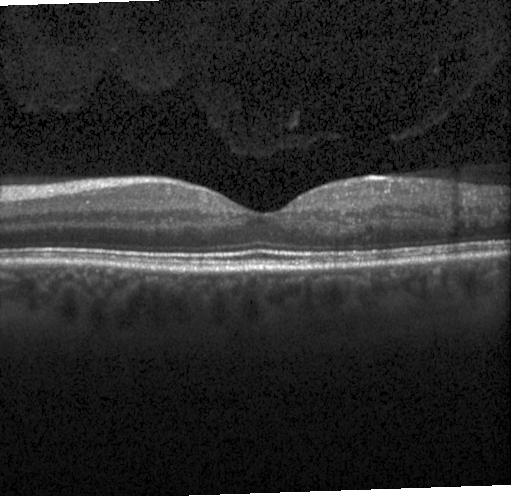 Impression: no evidence of choroidal neovascularization, diabetic macular edema, or drusen.